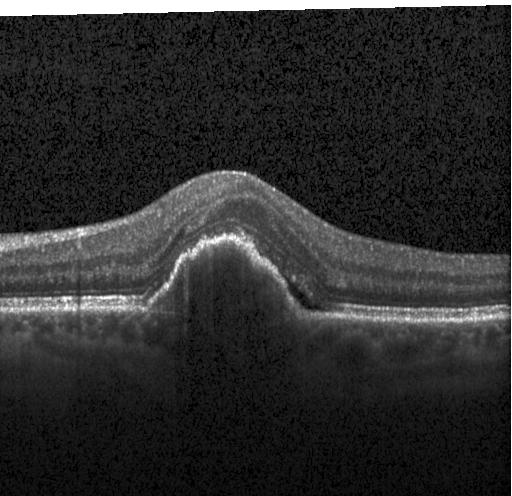
Diagnosis: a choroidal neovascular membrane.